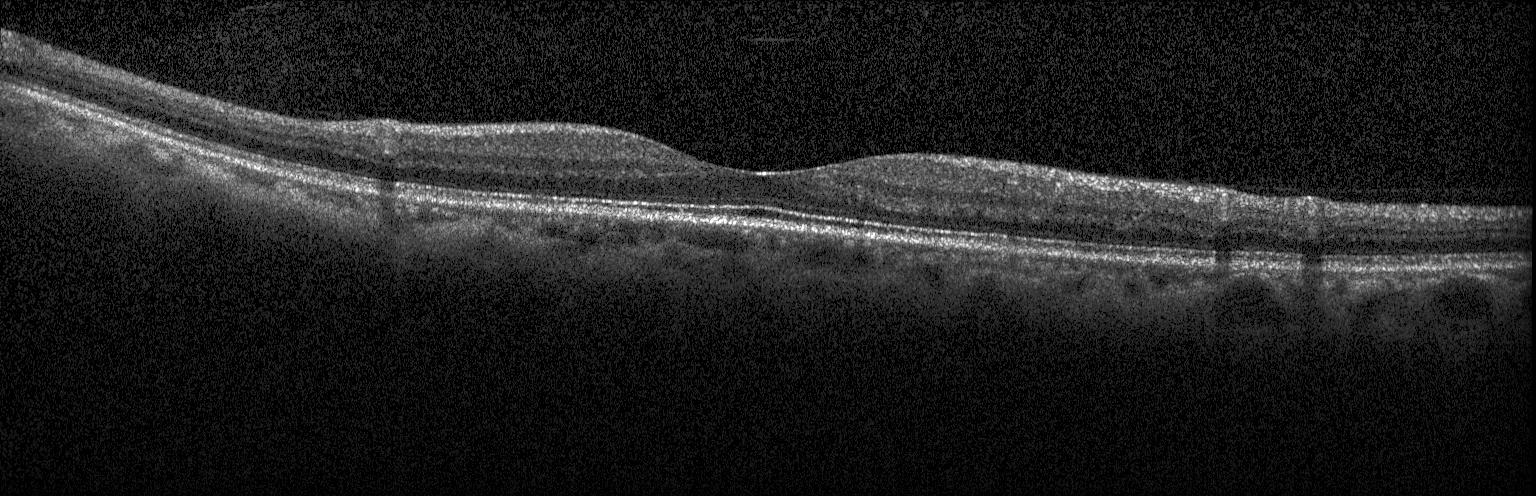 OCT finding: no evidence of choroidal neovascularization, diabetic macular edema, or drusen.